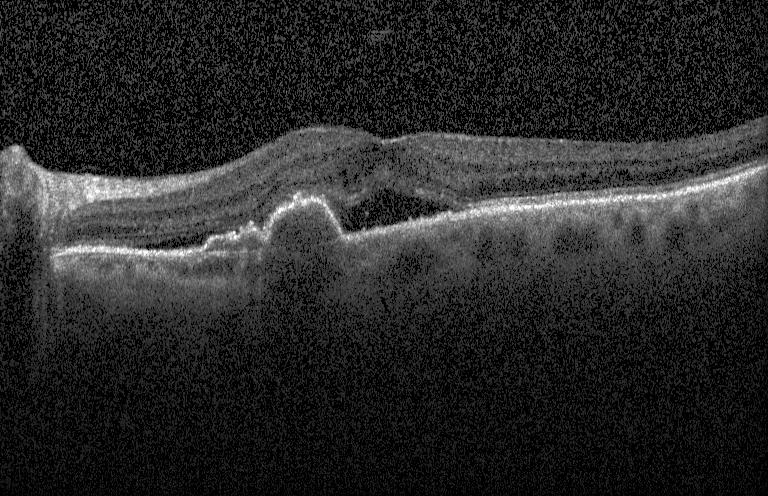
Retinal OCT cross-section; SD-OCT; Heidelberg Spectralis; through the macula — Impression: a choroidal neovascular membrane.